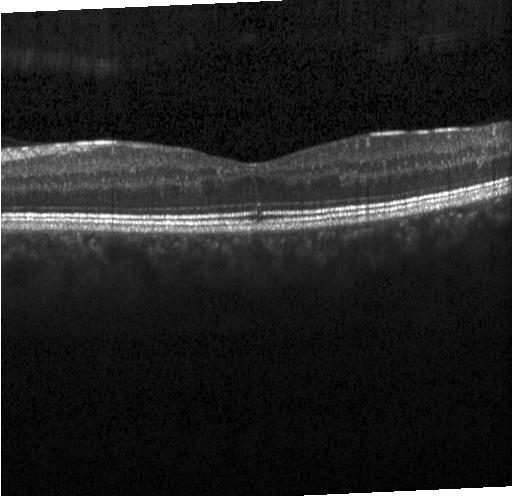
Dx: no choroidal neovascularization, no diabetic macular edema, and no drusen.